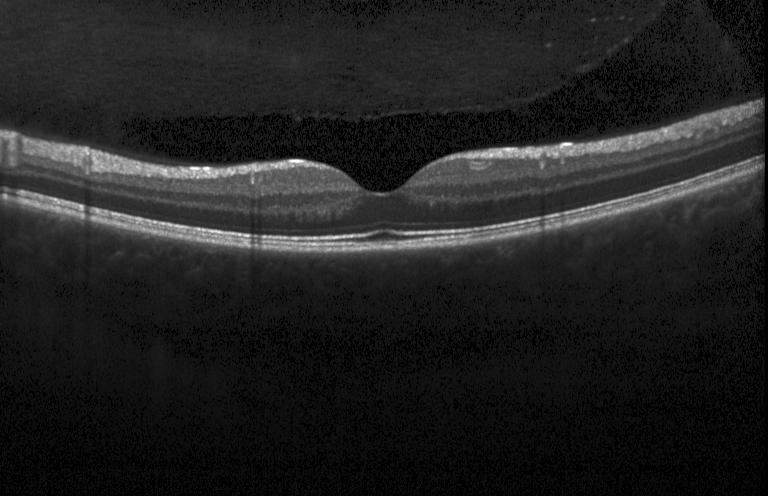 OCT finding: no choroidal neovascularization, no diabetic macular edema, and no drusen.